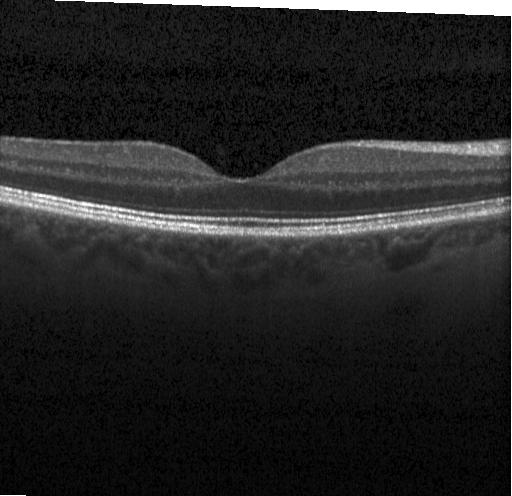
Centered on the fovea; instrument: Heidelberg Spectralis; OCT line scan; spectral-domain OCT. The scan shows no evidence of CNV, DME, or drusen.